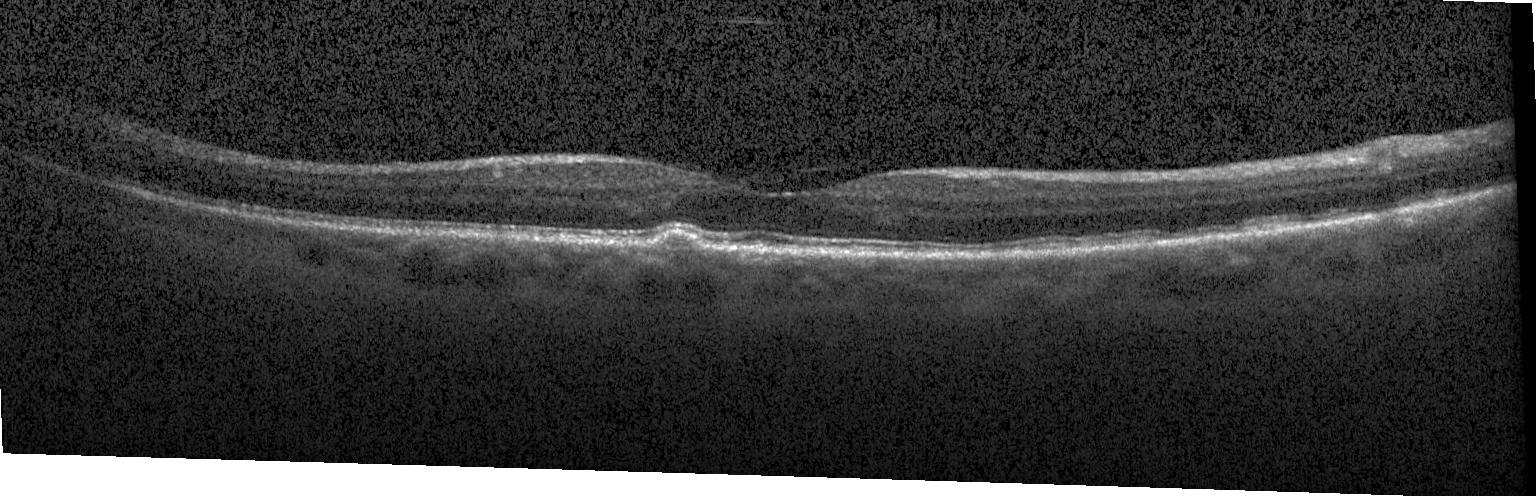
OCT finding: drusen.